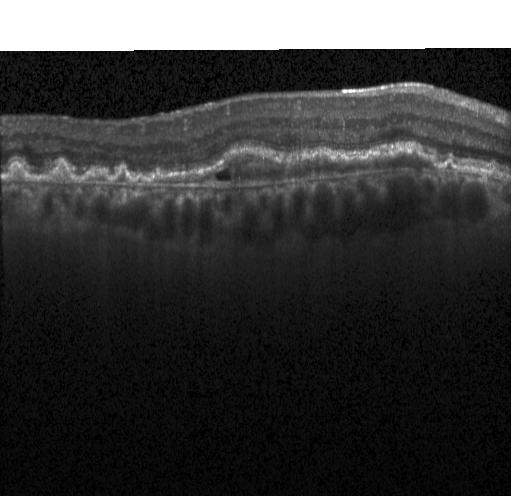

OCT scan showing choroidal neovascularization (CNV).